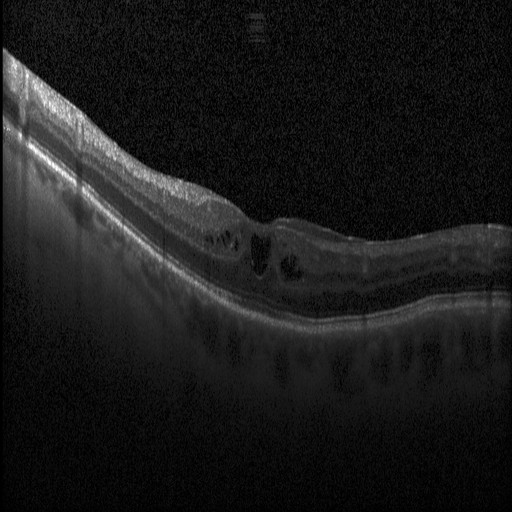

OCT B-scan.
Assessment: DME.